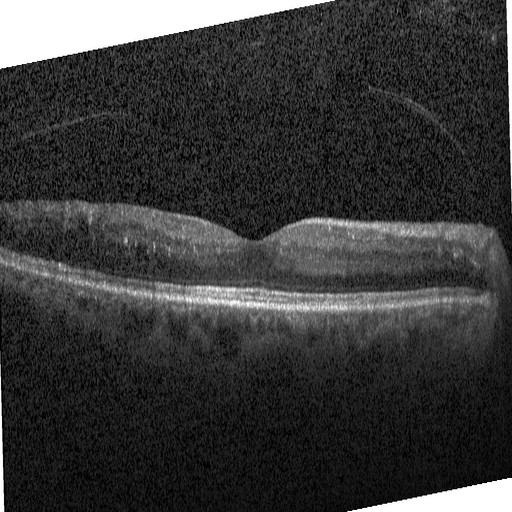
OCT B-scan.
Finding: DME.